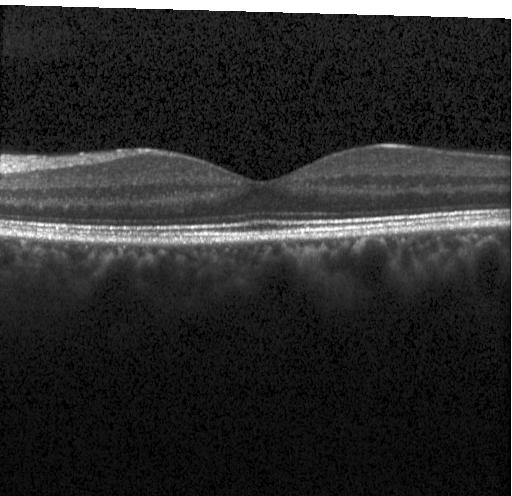
Finding: no choroidal neovascularization, diabetic macular edema, or drusen.